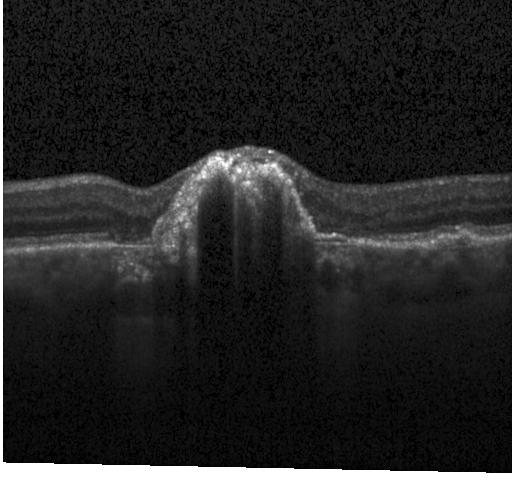

Macular OCT demonstrating a choroidal neovascular membrane.